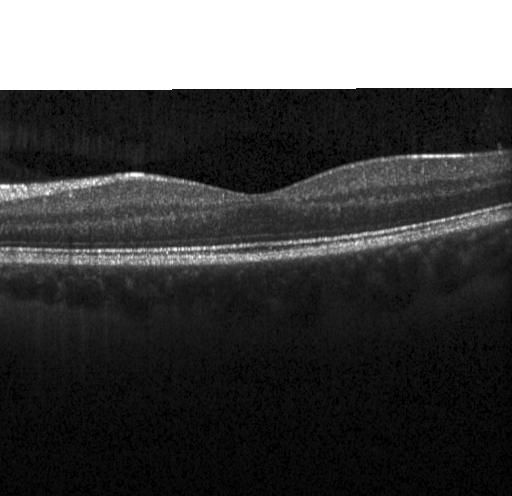 Fovea-centered; SD-OCT; acquired on a Heidelberg Spectralis; optical coherence tomography B-scan
Diagnosis: no choroidal neovascularization, no diabetic macular edema, and no drusen.